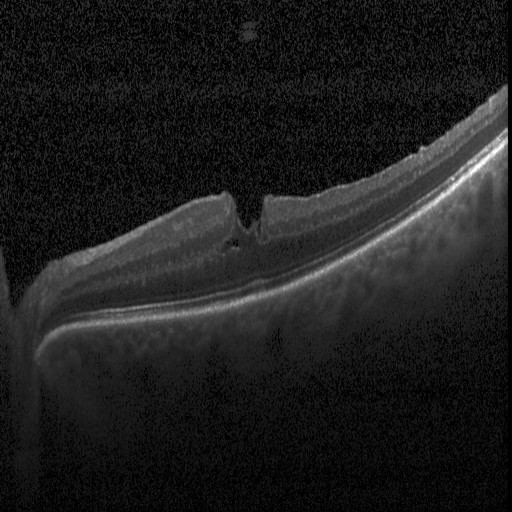
Instrument: Heidelberg Spectralis, optical coherence tomography scan. Impression: diabetic macular edema (DME).